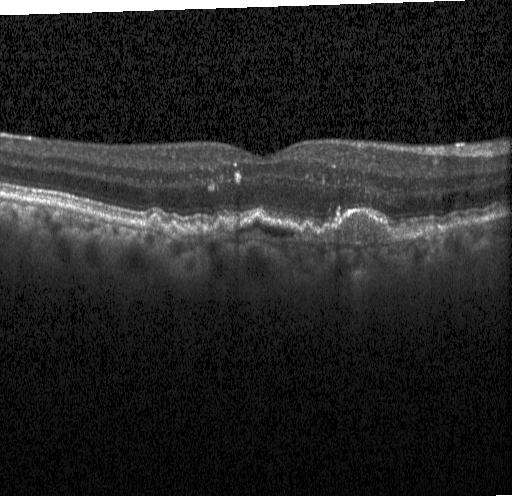 Centered on the fovea · Heidelberg Spectralis · SD-OCT · optical coherence tomography B-scan — This B-scan demonstrates a choroidal neovascular membrane.